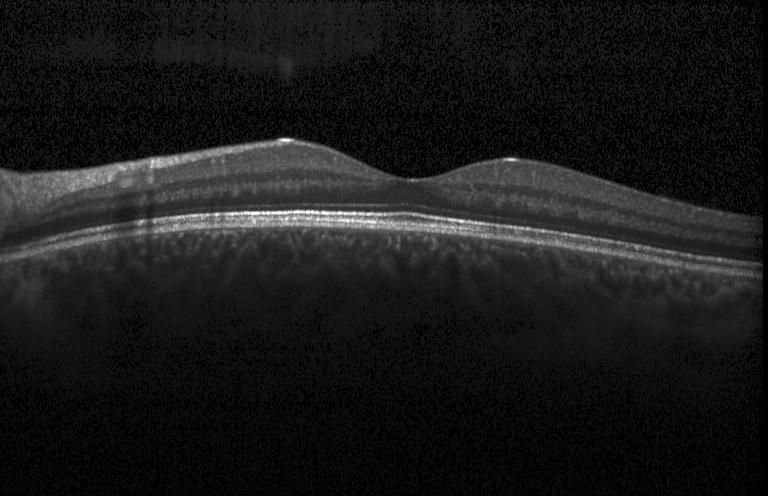

Through the macula. OCT line scan — This B-scan demonstrates no CNV, no DME, and no drusen.